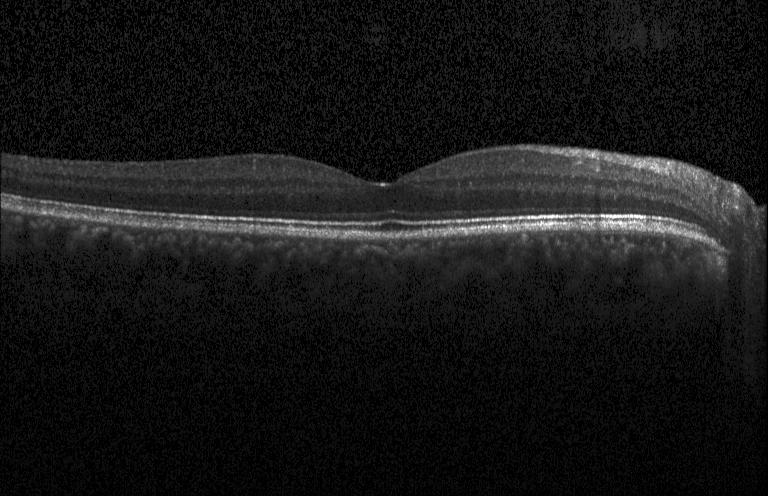

Optical coherence tomography scan.
No CNV, DME, or drusen.